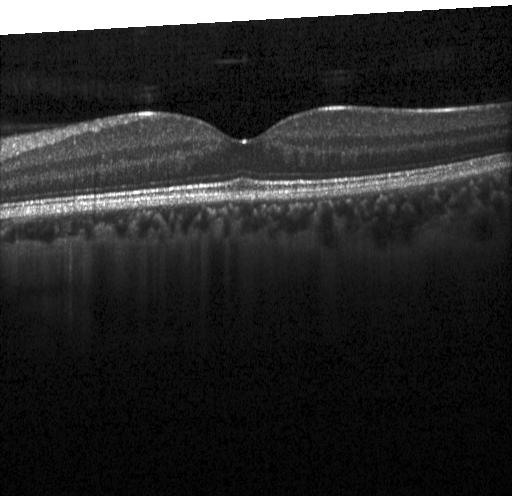 Acquired on a Heidelberg Spectralis; OCT B-scan; centered on the fovea. Diagnosis: no choroidal neovascularization, diabetic macular edema, or drusen.